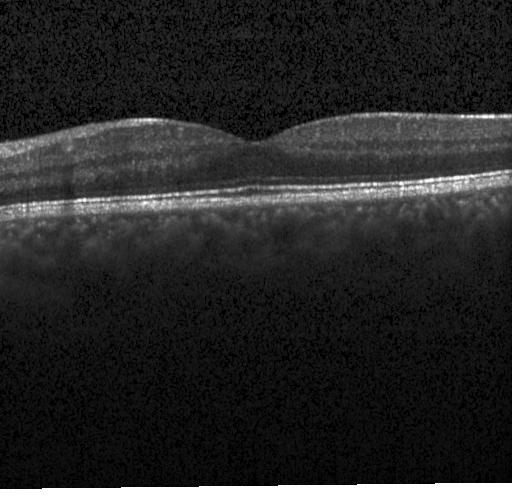 Finding: neither choroidal neovascularization, diabetic macular edema, nor drusen.